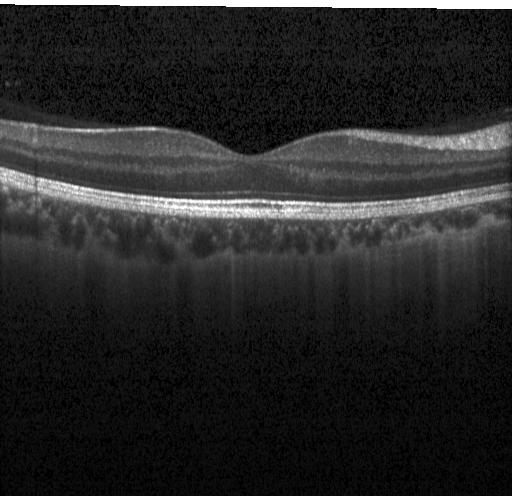
OCT B-scan — Macular OCT: no choroidal neovascularization, no diabetic macular edema, and no drusen.